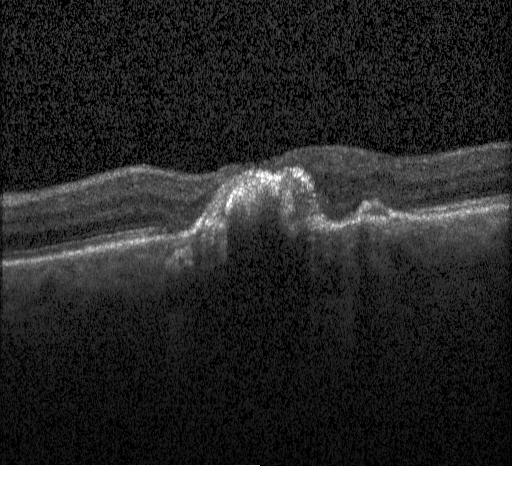

Fovea-centered, retinal OCT B-scan, SD-OCT. Impression: a choroidal neovascular membrane.